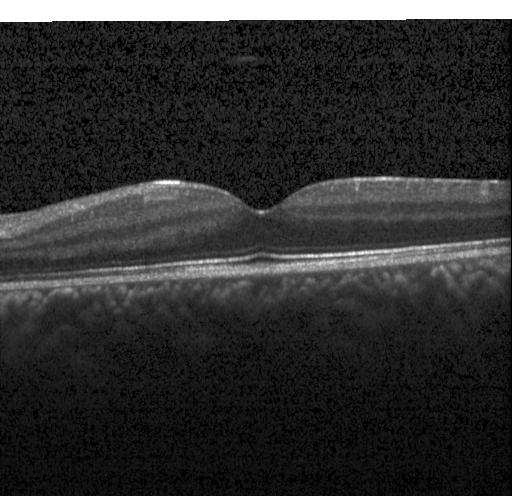 Dx: no choroidal neovascularization, no diabetic macular edema, and no drusen.